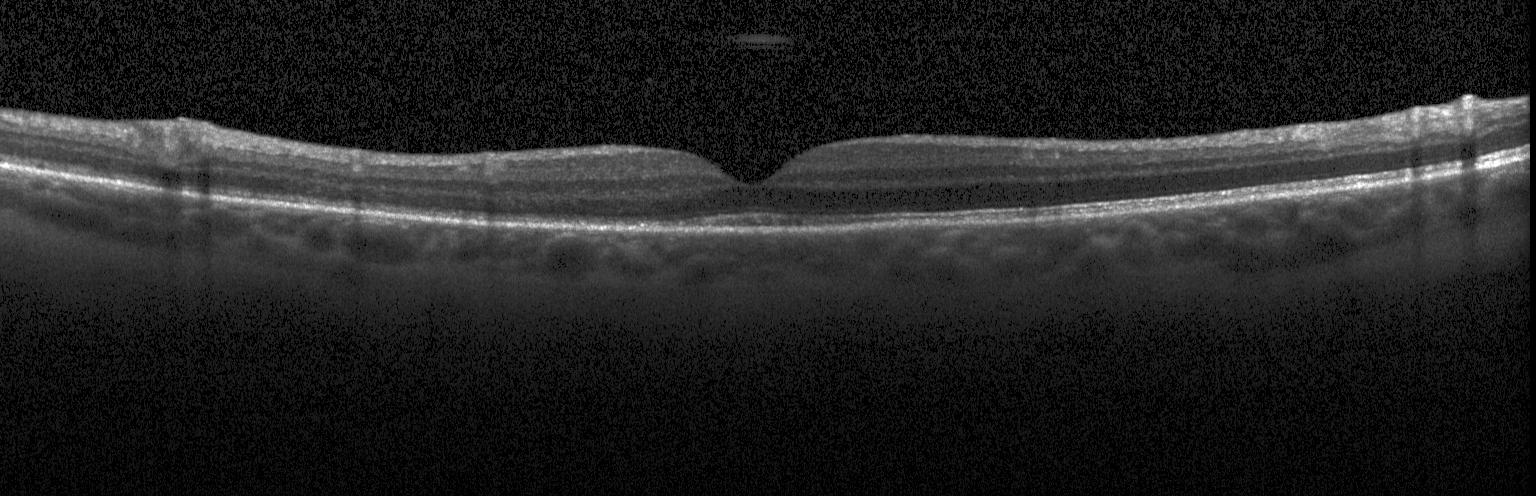

Retinal OCT B-scan. The scan shows neither choroidal neovascularization, diabetic macular edema, nor drusen.